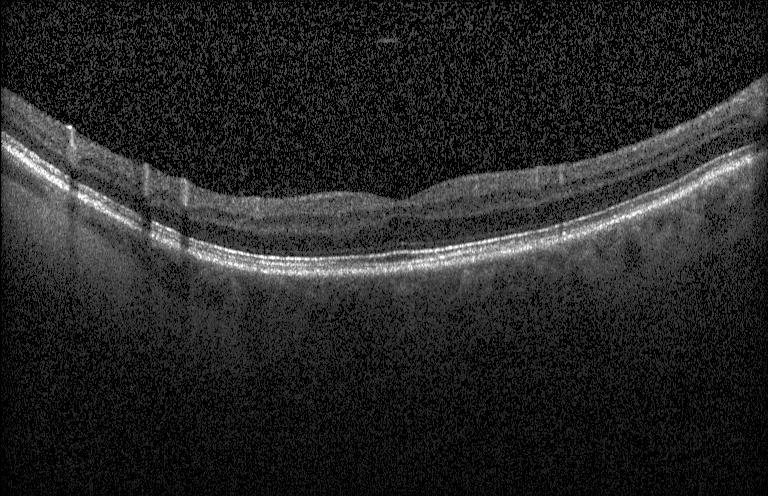

Retinal OCT cross-section showing neither CNV, DME, nor drusen.